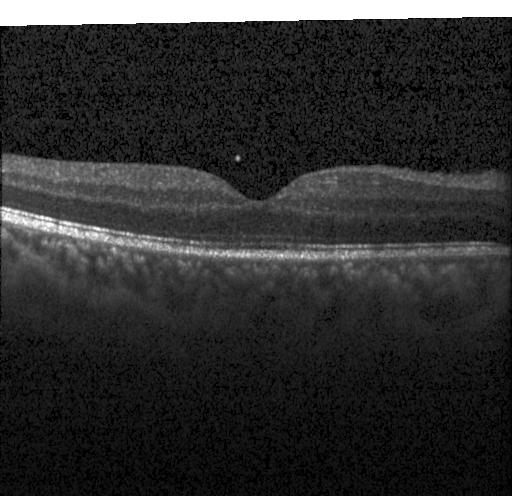
Retinal OCT cross-section showing no choroidal neovascularization, no diabetic macular edema, and no drusen.